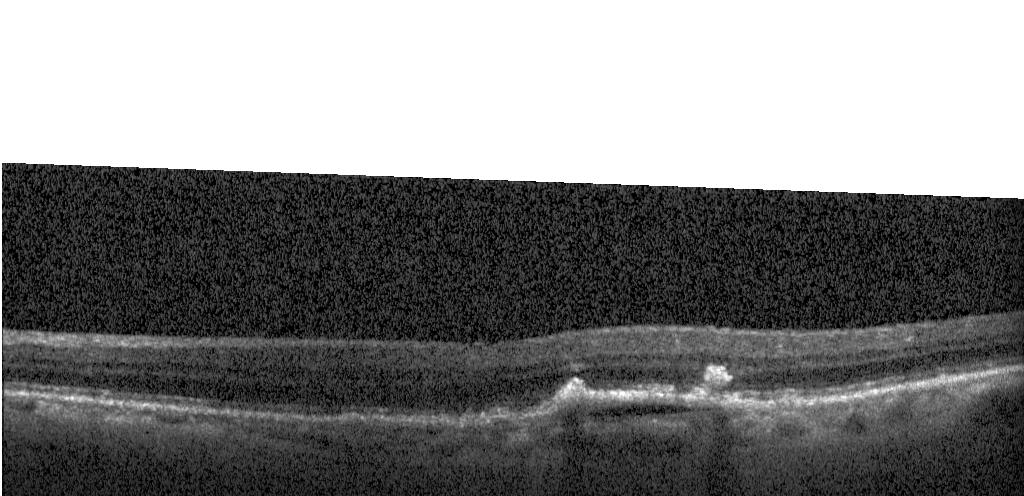 Heidelberg Spectralis, through the macula, SD-OCT, retinal OCT B-scan — The scan shows choroidal neovascularization (CNV).